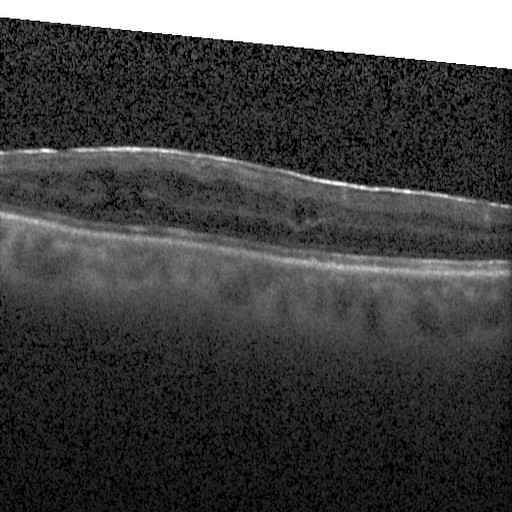
DME.